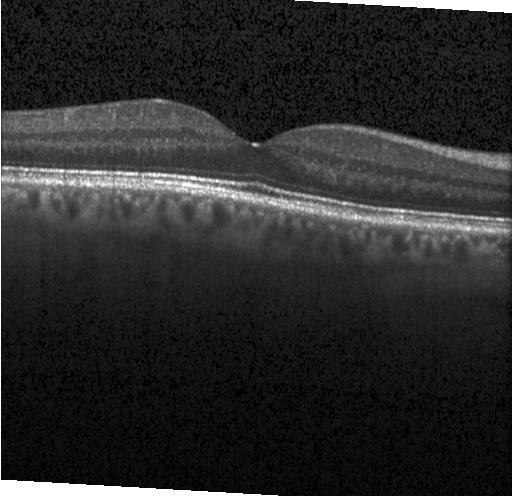
Assessment: no evidence of CNV, DME, or drusen.